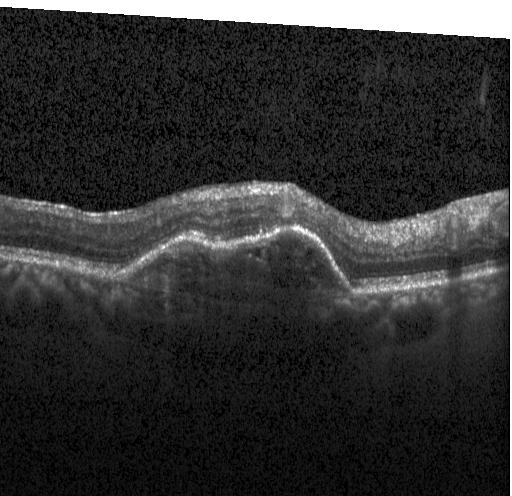 Retinal OCT B-scan. The scan shows choroidal neovascularization (CNV).